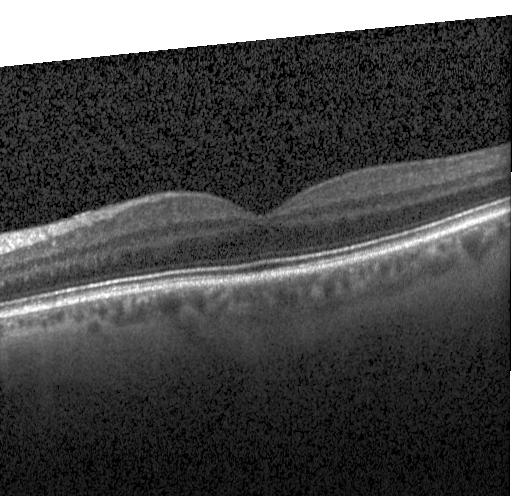

Spectral-domain OCT. Instrument: Heidelberg Spectralis. OCT B-scan
Dx: no choroidal neovascularization, no diabetic macular edema, and no drusen.